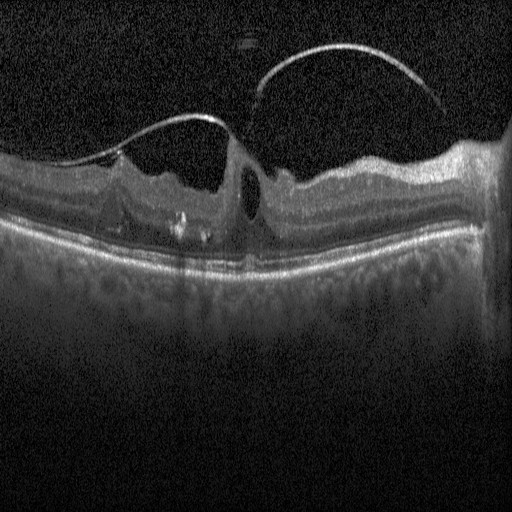
Spectral-domain OCT. Horizontal scan through the fovea. Optical coherence tomography B-scan — Dx: DME.